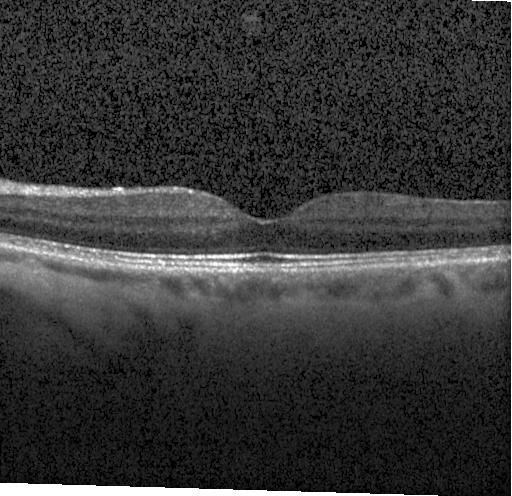 Retinal OCT B-scan · instrument: Heidelberg Spectralis
This B-scan demonstrates no choroidal neovascularization, diabetic macular edema, or drusen.